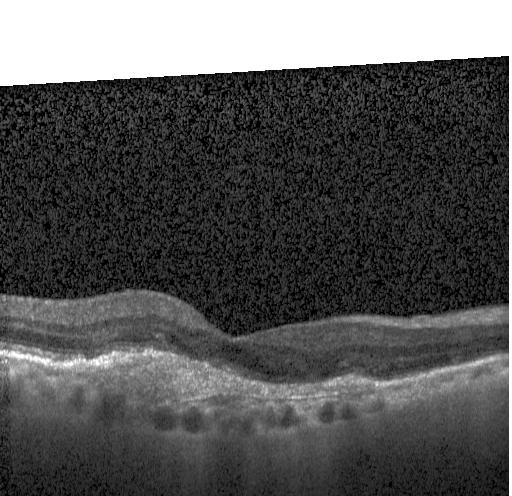
Optical coherence tomography scan — OCT finding: a choroidal neovascular membrane.